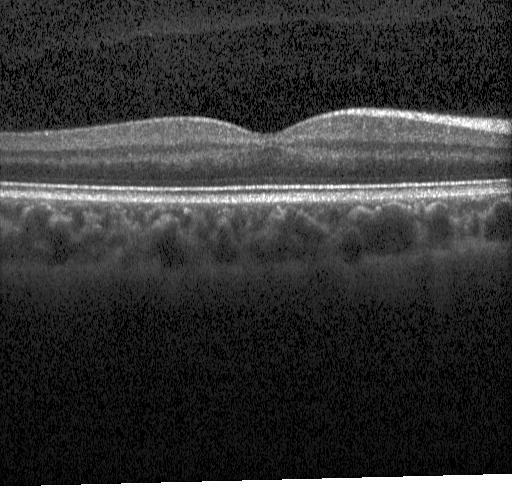

OCT B-scan — The scan shows no evidence of choroidal neovascularization, diabetic macular edema, or drusen.